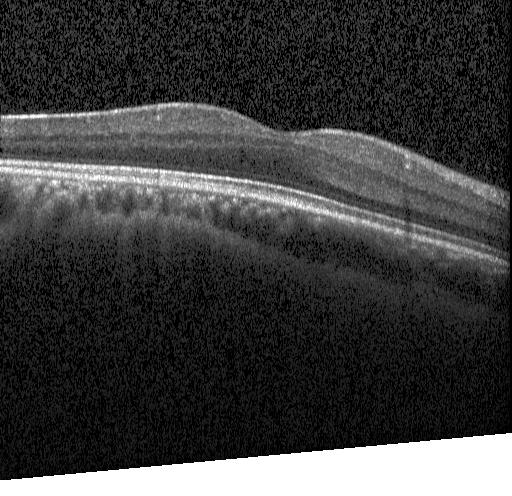

OCT line scan
This B-scan demonstrates neither choroidal neovascularization, diabetic macular edema, nor drusen.